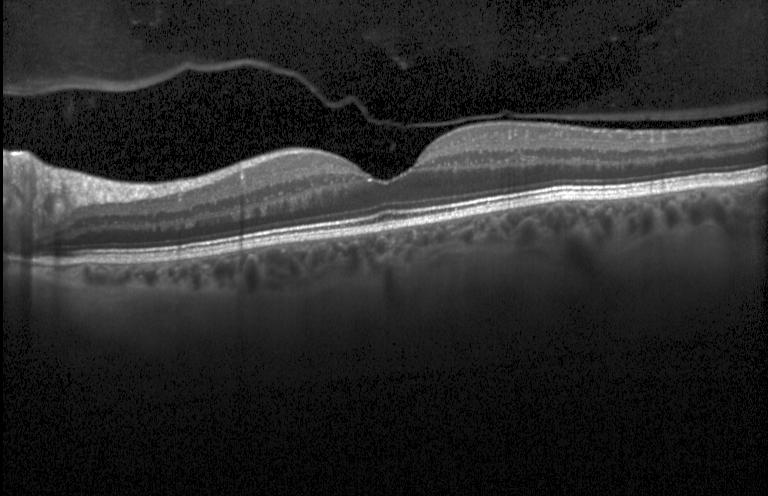
OCT B-scan, instrument: Heidelberg Spectralis — Finding: no evidence of choroidal neovascularization, diabetic macular edema, or drusen.